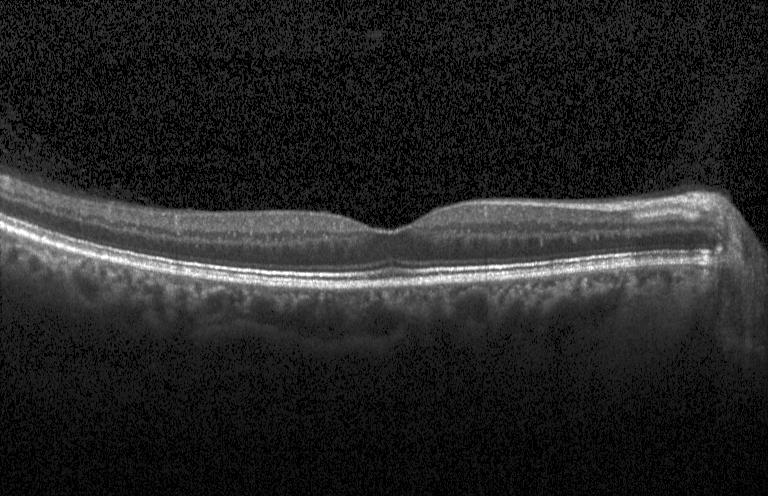
Optical coherence tomography scan, SD-OCT. No choroidal neovascularization, no diabetic macular edema, and no drusen.